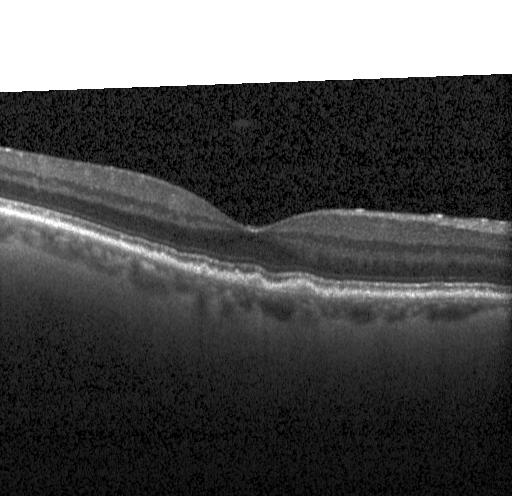

Optical coherence tomography scan · horizontal scan through the fovea · spectral-domain optical coherence tomography
OCT finding: drusen.